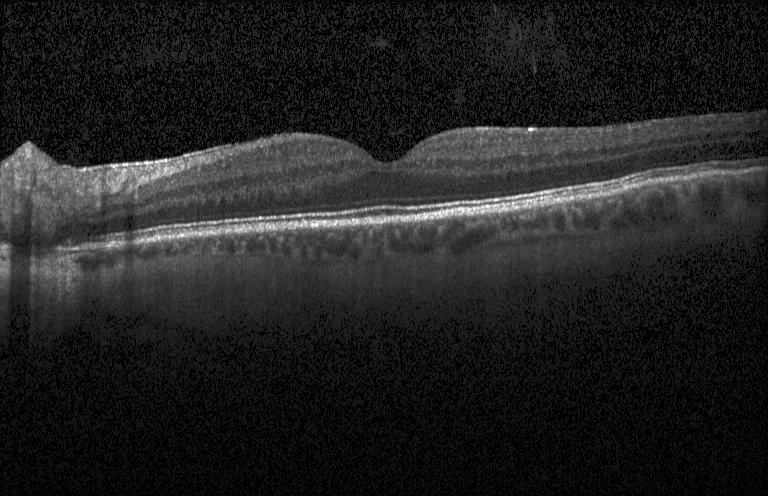

Macular OCT demonstrating neither choroidal neovascularization, diabetic macular edema, nor drusen.